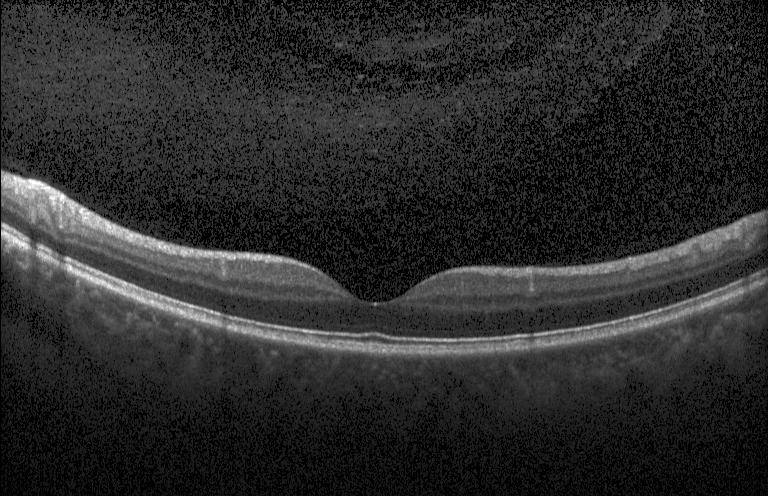

Finding: no evidence of choroidal neovascularization, diabetic macular edema, or drusen.